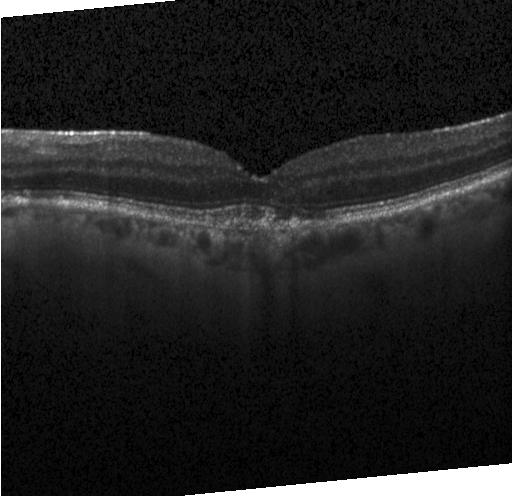
Optical coherence tomography B-scan. SD-OCT — Dx: a choroidal neovascular membrane.